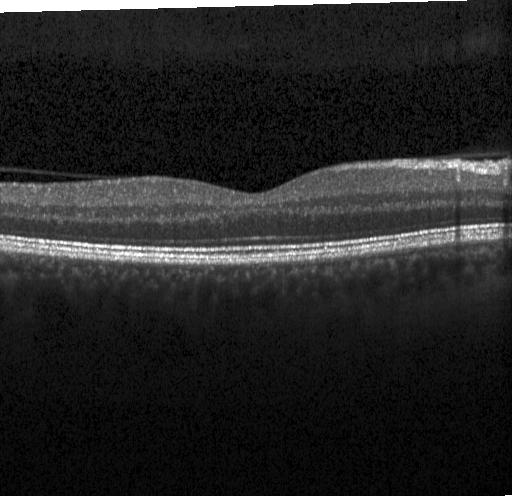 SD-OCT. Retinal OCT B-scan. Centered on the fovea. The scan shows neither choroidal neovascularization, diabetic macular edema, nor drusen.